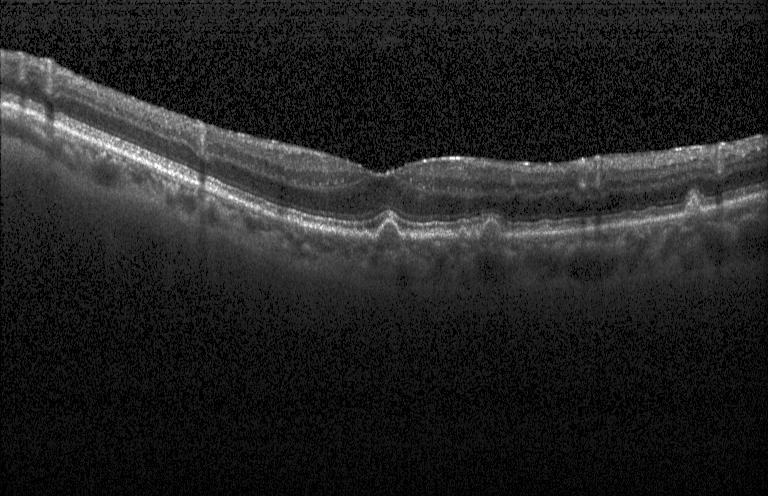

Optical coherence tomography B-scan, horizontal scan through the fovea, spectral-domain optical coherence tomography.
Drusen.